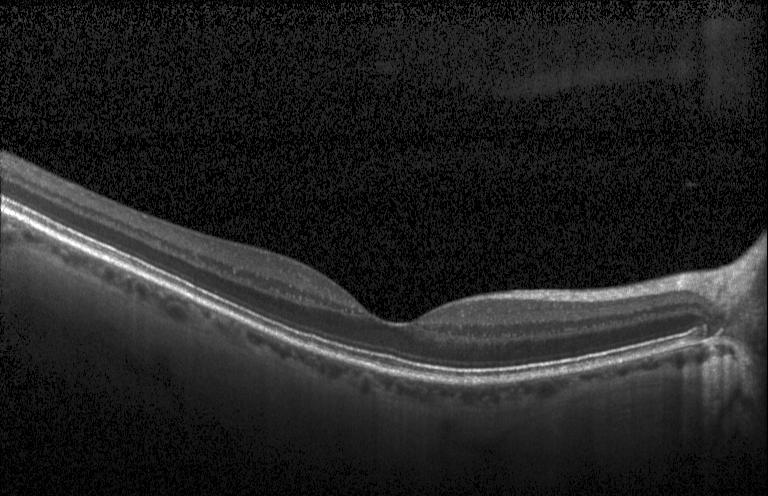

OCT B-scan · SD-OCT · fovea-centered · Heidelberg Spectralis OCT system.
This B-scan demonstrates no CNV, DME, or drusen.